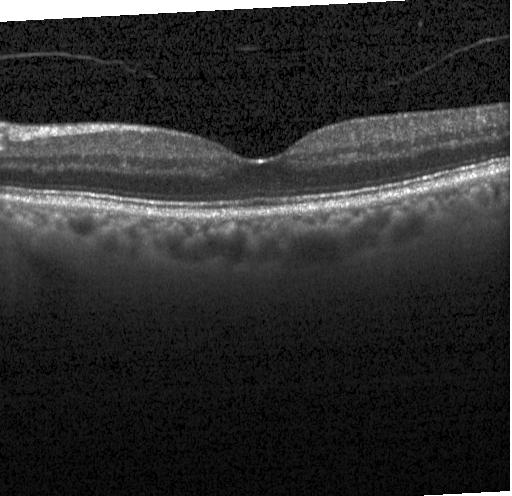
Impression: neither choroidal neovascularization, diabetic macular edema, nor drusen.